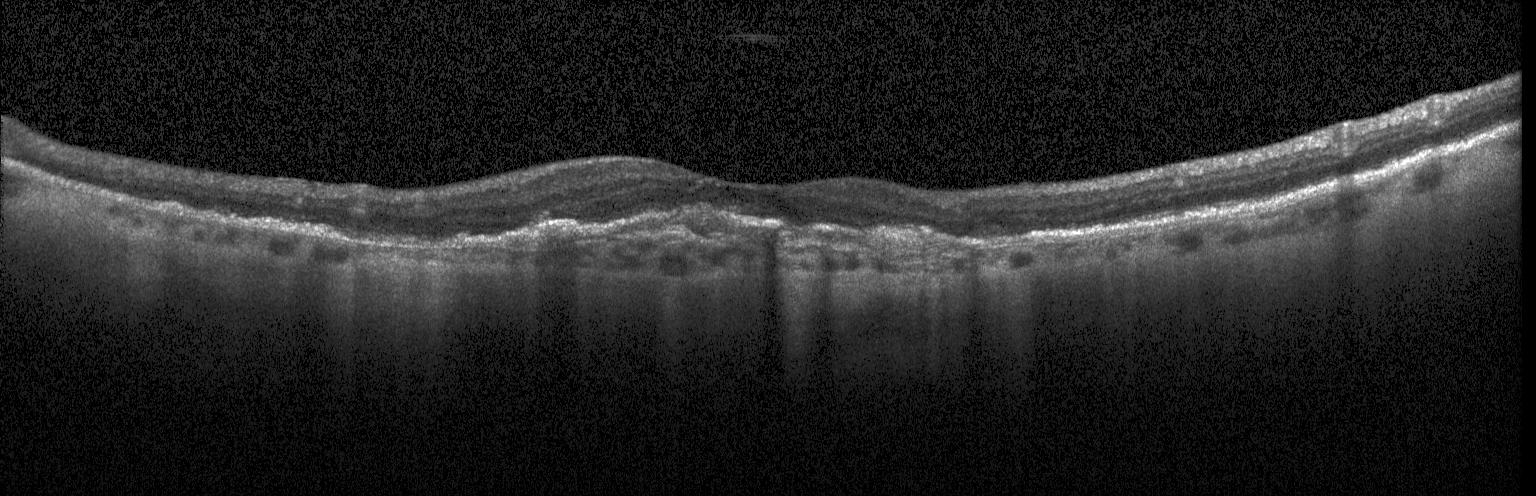 Retinal OCT cross-section · fovea-centered. Assessment: a choroidal neovascular membrane.